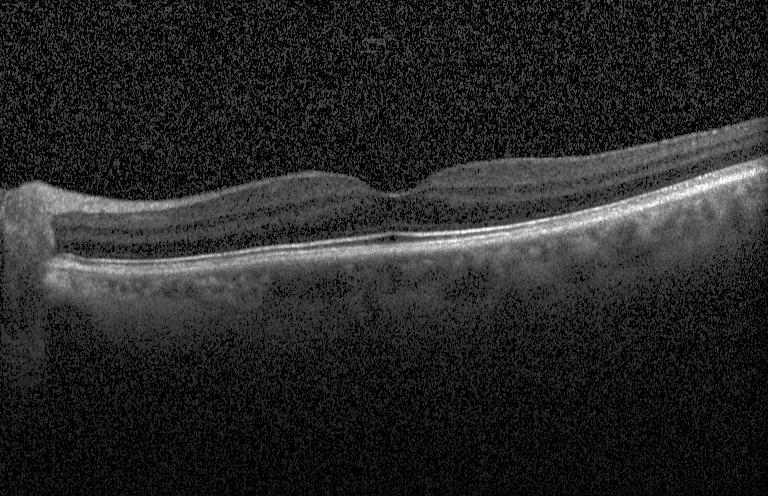 Dx: no choroidal neovascularization, diabetic macular edema, or drusen.